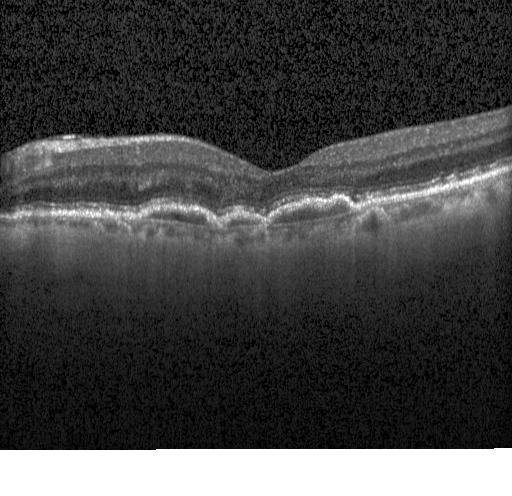 OCT B-scan · through the macula · Heidelberg Spectralis OCT system.
Finding: choroidal neovascularization (CNV).